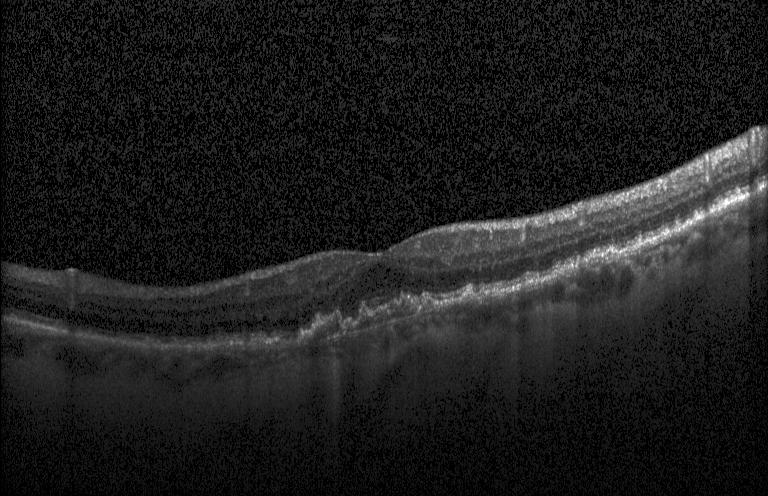 Retinal OCT cross-section · fovea-centered · Heidelberg Spectralis OCT system · spectral-domain OCT. A choroidal neovascular membrane.